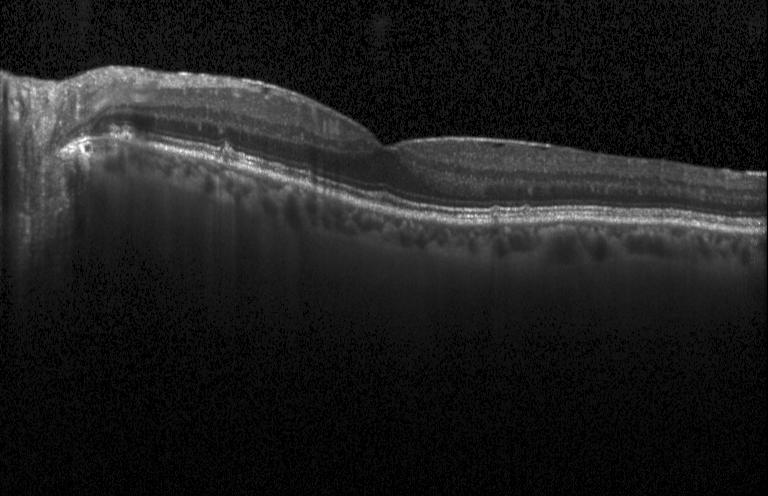
Assessment: multiple drusen.